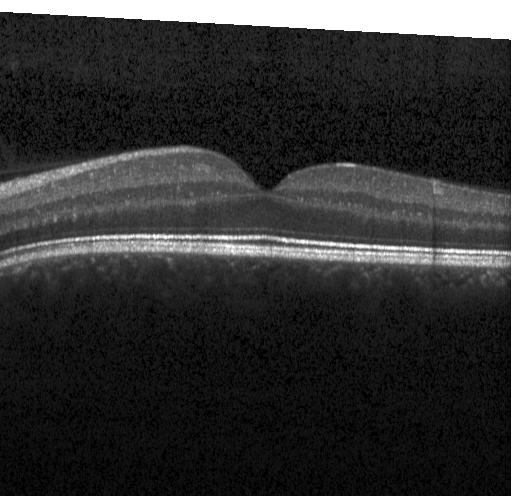 Spectral-domain OCT B-scan: no CNV, no DME, and no drusen.